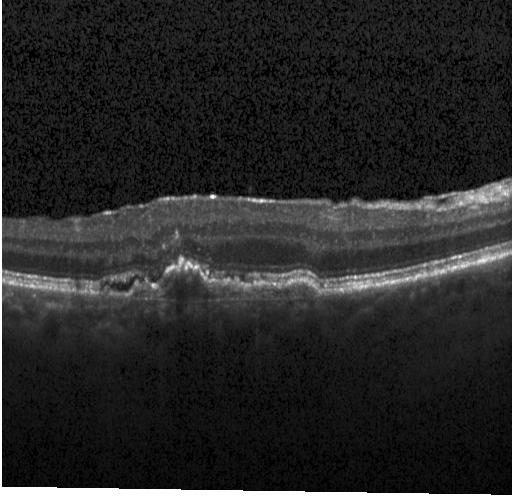 Impression: CNV.